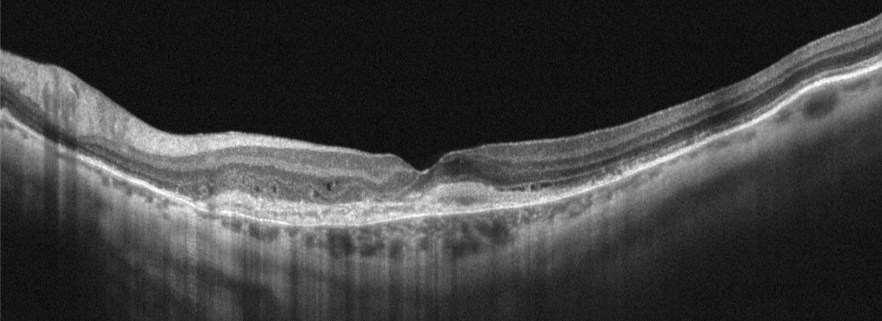
Impression: AMD.